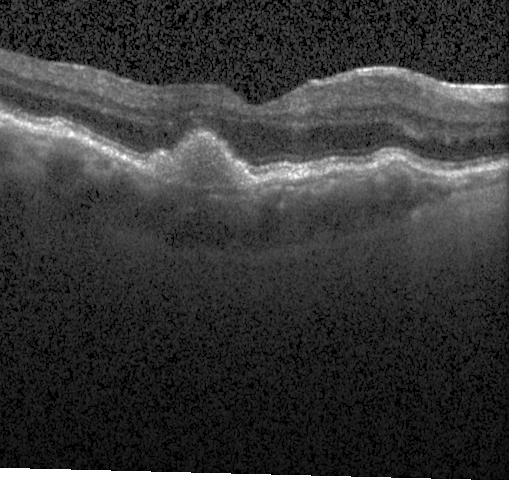 OCT scan showing a choroidal neovascular membrane.